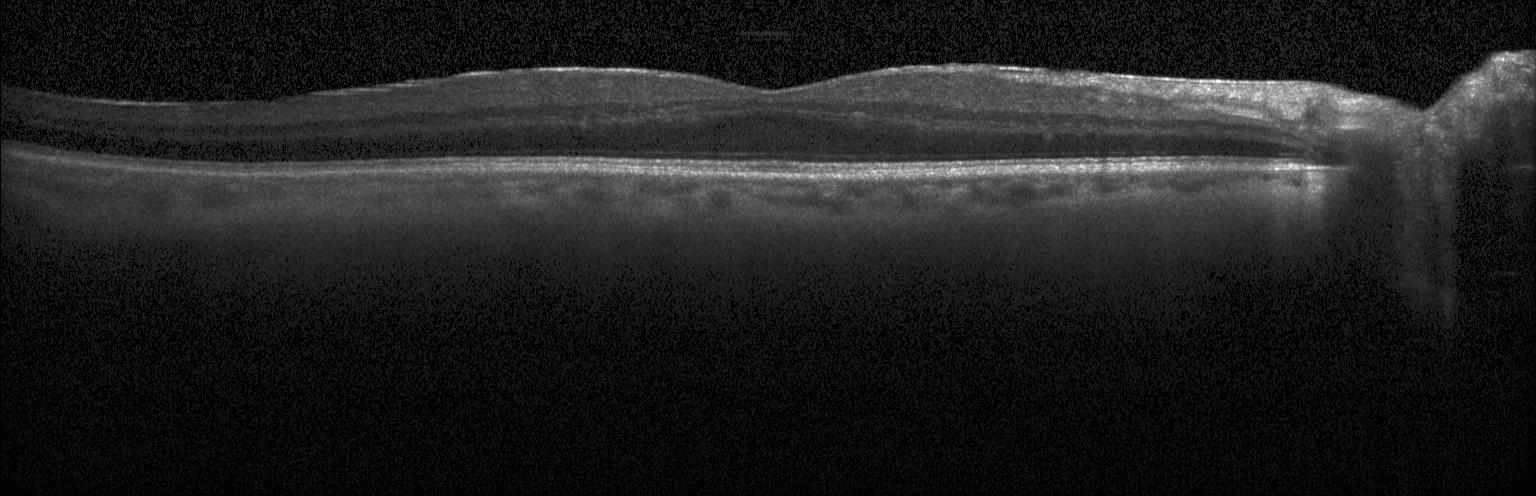 Centered on the fovea; acquired on a Heidelberg Spectralis; OCT line scan; SD-OCT.
OCT finding: no choroidal neovascularization, diabetic macular edema, or drusen.